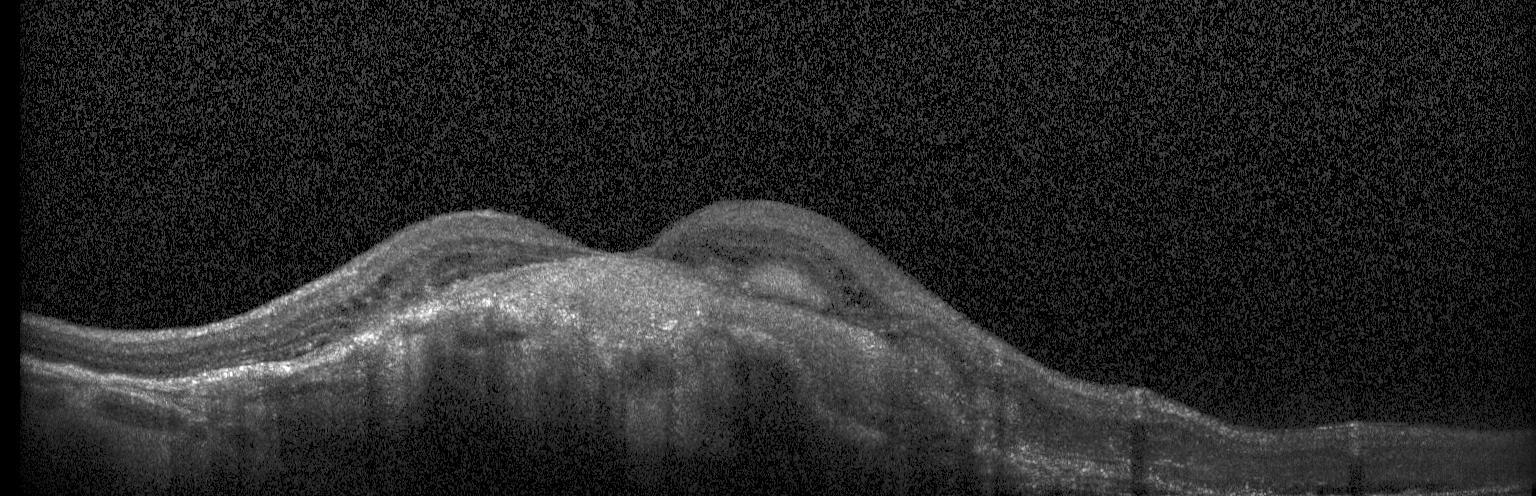

OCT B-scan. Finding: CNV.